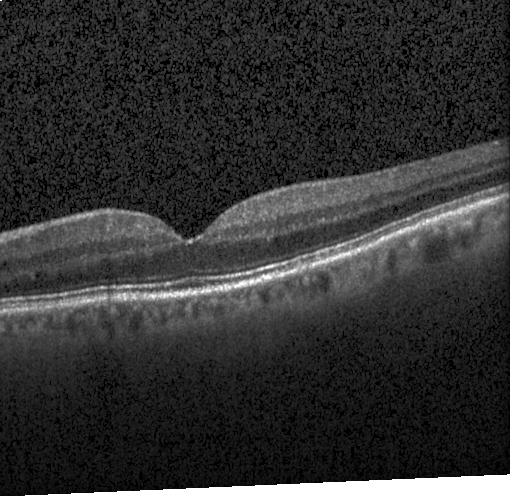 Heidelberg Spectralis. Optical coherence tomography scan. Spectral-domain OCT
Impression: neither choroidal neovascularization, diabetic macular edema, nor drusen.